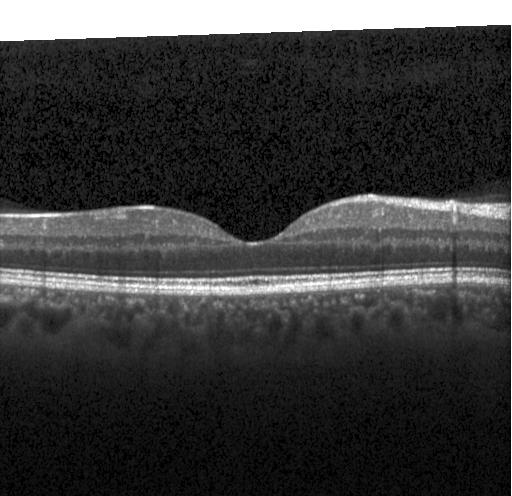

Heidelberg Spectralis OCT system. Retinal OCT cross-section. Finding: neither choroidal neovascularization, diabetic macular edema, nor drusen.